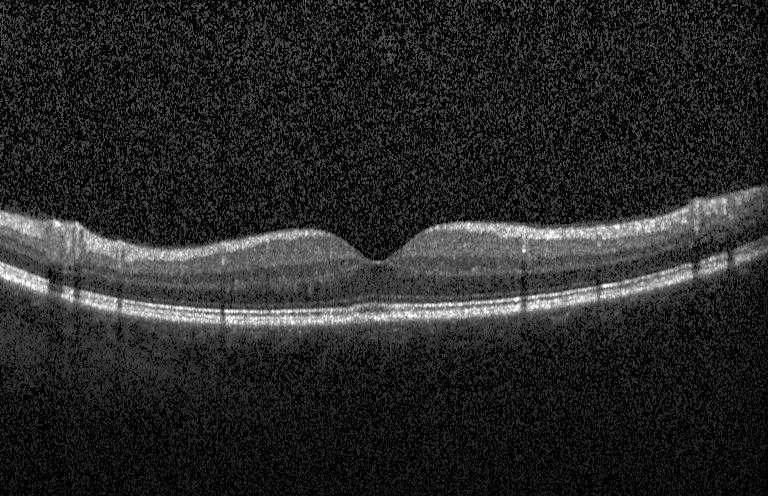

OCT B-scan showing no choroidal neovascularization, diabetic macular edema, or drusen.